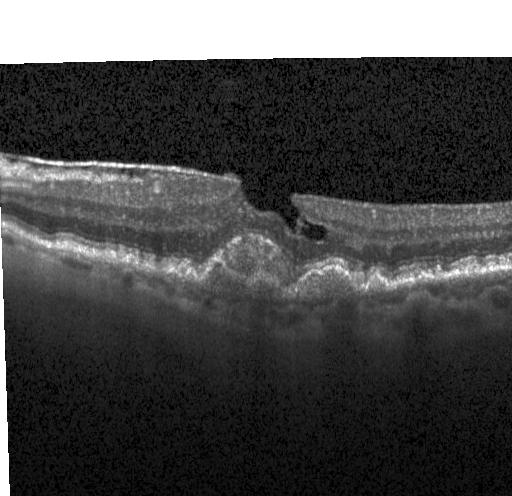
Horizontal scan through the fovea, OCT B-scan, acquired on a Heidelberg Spectralis, spectral-domain optical coherence tomography — Impression: a choroidal neovascular membrane.